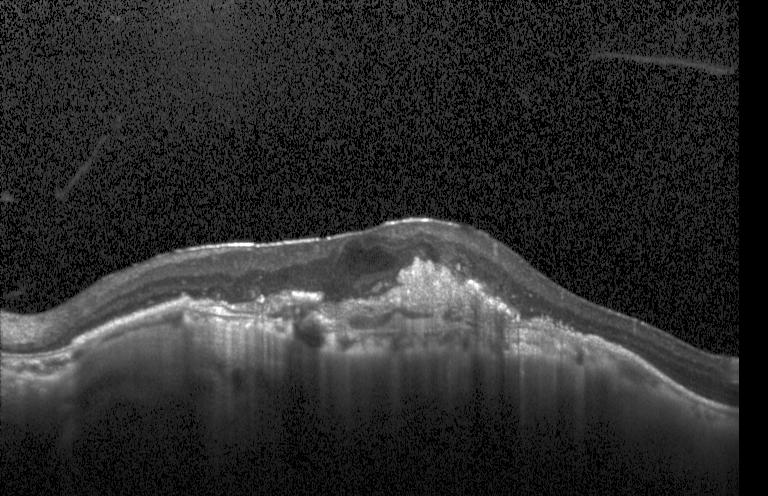

Macular OCT: a choroidal neovascular membrane.